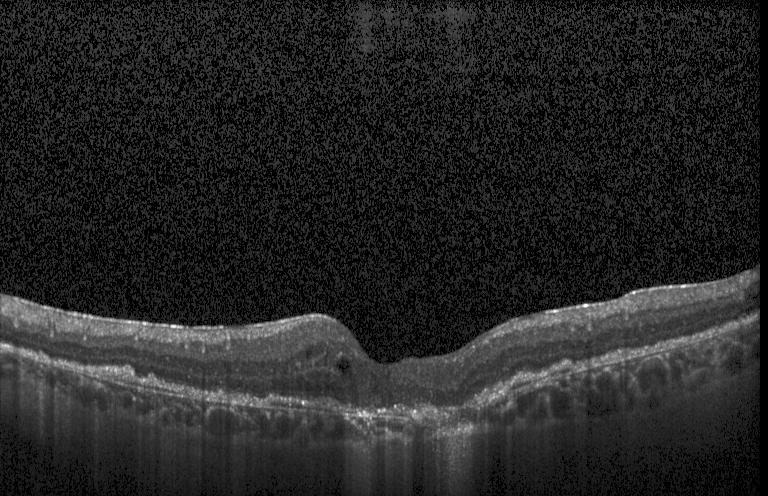
Optical coherence tomography scan — Finding: a choroidal neovascular membrane.